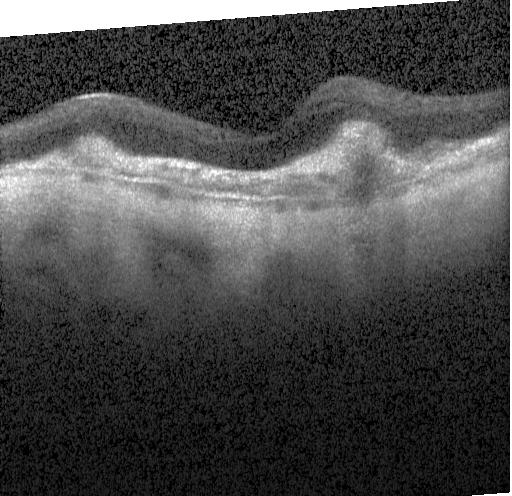 The scan shows a choroidal neovascular membrane.